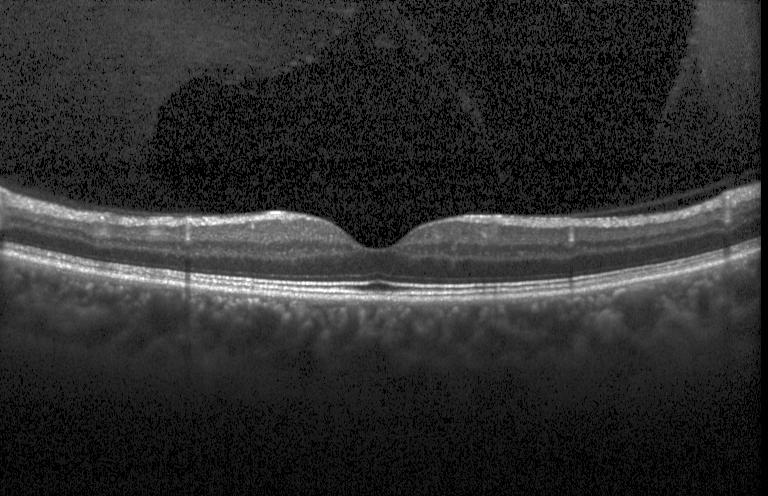

OCT finding: neither choroidal neovascularization, diabetic macular edema, nor drusen.